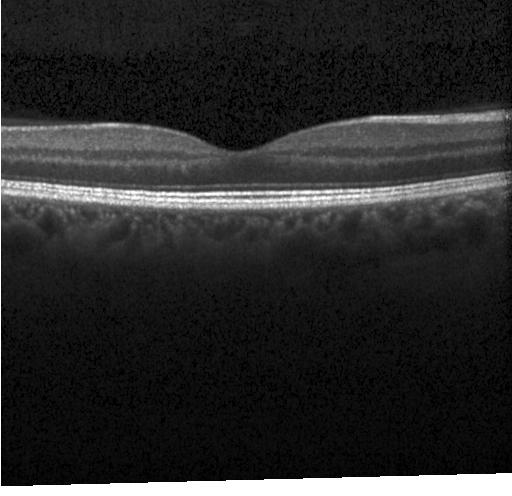
Heidelberg Spectralis OCT system · retinal OCT cross-section · horizontal scan through the fovea.
Dx: neither CNV, DME, nor drusen.